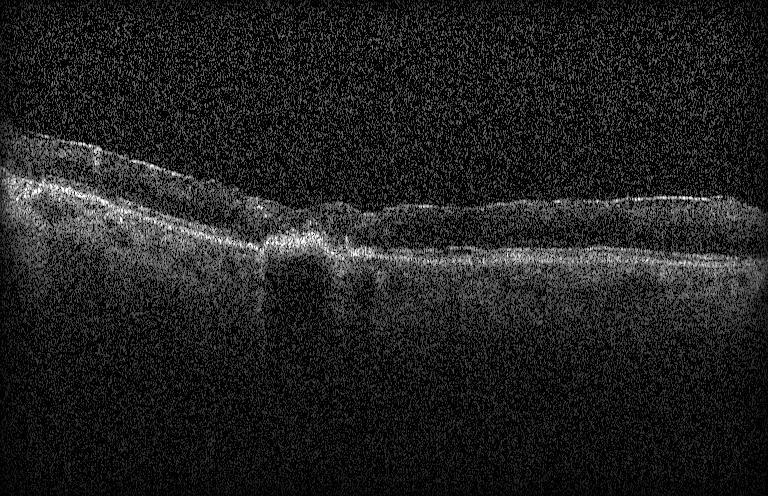
Spectral-domain optical coherence tomography · Heidelberg Spectralis OCT system · OCT B-scan · macular scan
OCT finding: choroidal neovascularization.